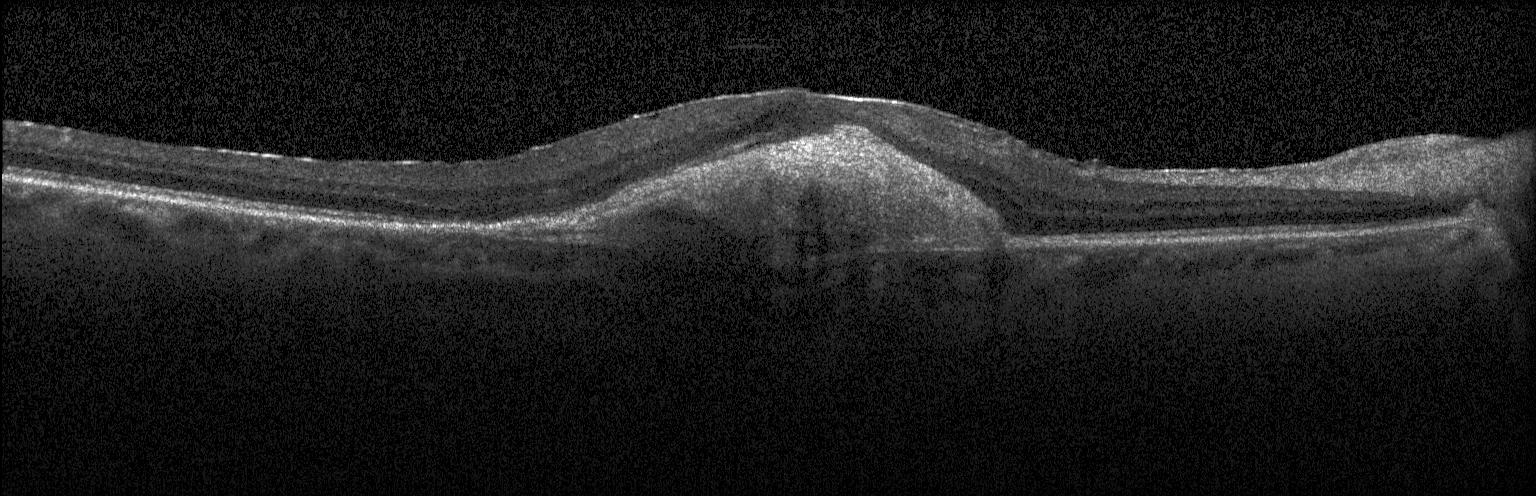
OCT B-scan — Impression: CNV.